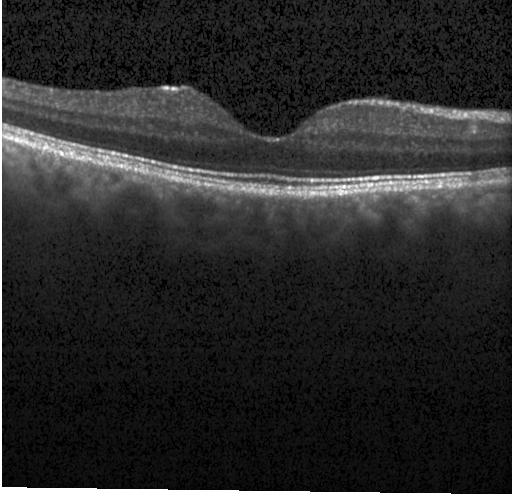 Retinal OCT B-scan · acquired on a Heidelberg Spectralis · spectral-domain optical coherence tomography · through the macula — Impression: no choroidal neovascularization, no diabetic macular edema, and no drusen.